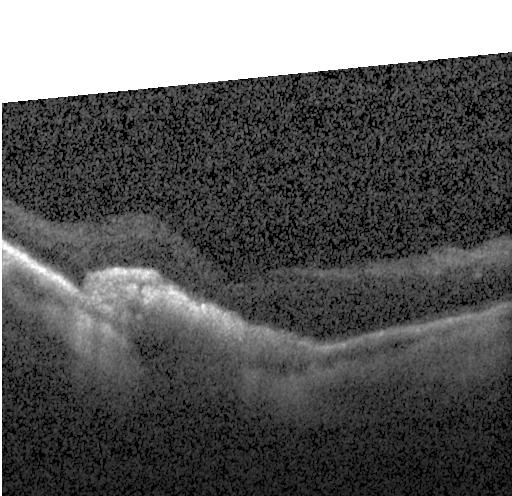

Optical coherence tomography scan.
Finding: a choroidal neovascular membrane.